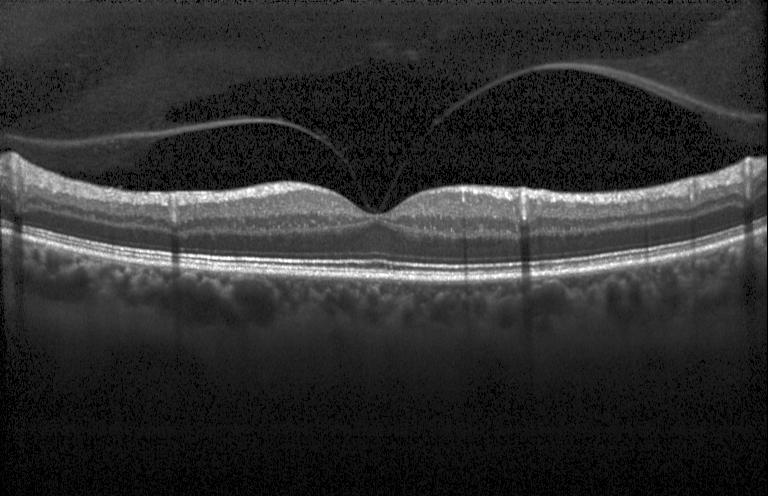 Finding: no choroidal neovascularization, diabetic macular edema, or drusen.